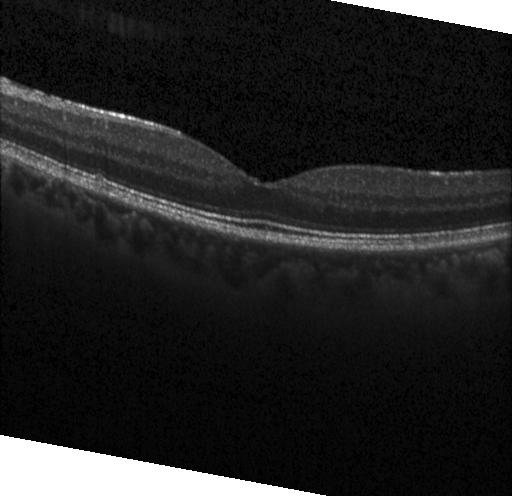
Finding: neither CNV, DME, nor drusen.